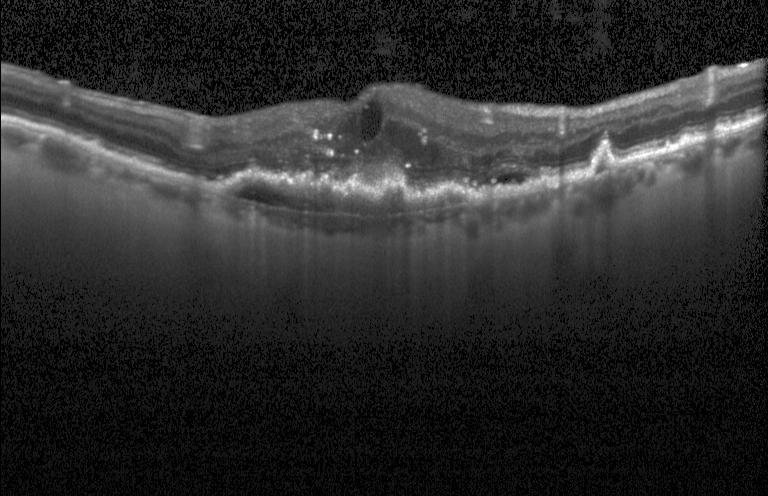 Retinal OCT cross-section. Dx: choroidal neovascularization.